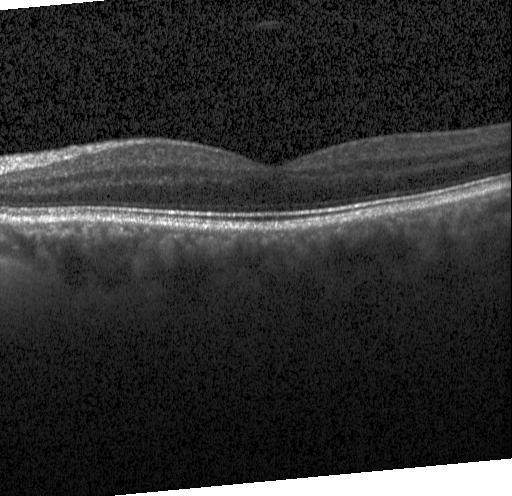
Through the macula · retinal OCT cross-section · spectral-domain optical coherence tomography · Heidelberg Spectralis. Finding: neither choroidal neovascularization, diabetic macular edema, nor drusen.